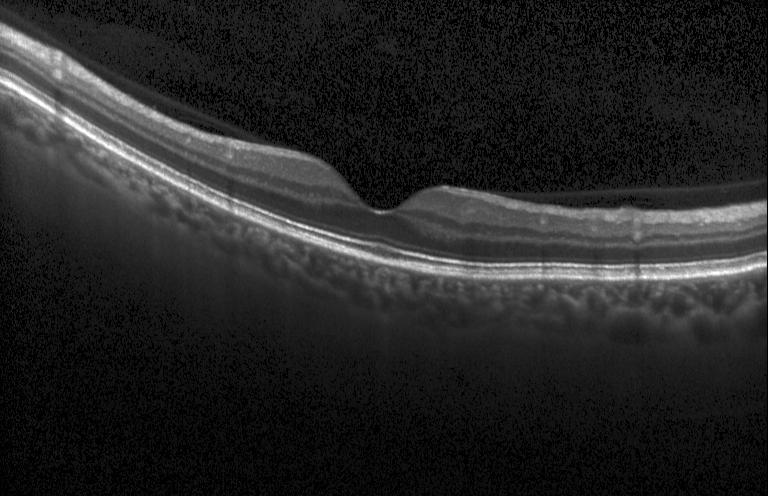 OCT line scan.
Assessment: no evidence of choroidal neovascularization, diabetic macular edema, or drusen.